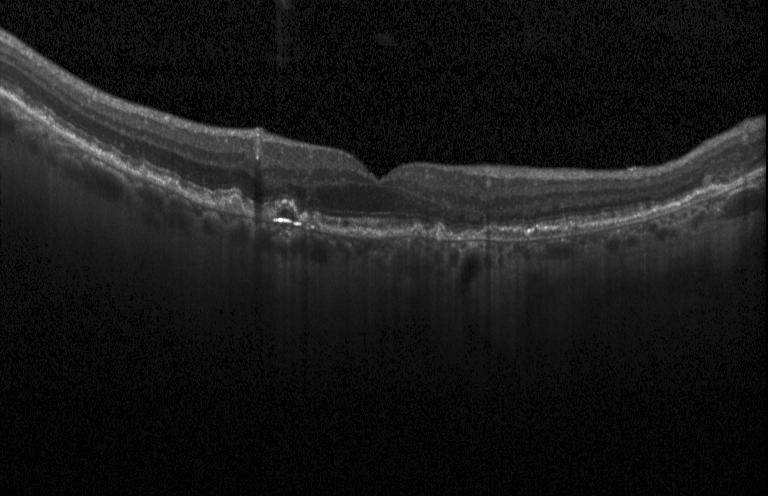
Optical coherence tomography B-scan, spectral-domain optical coherence tomography.
This B-scan demonstrates a choroidal neovascular membrane.